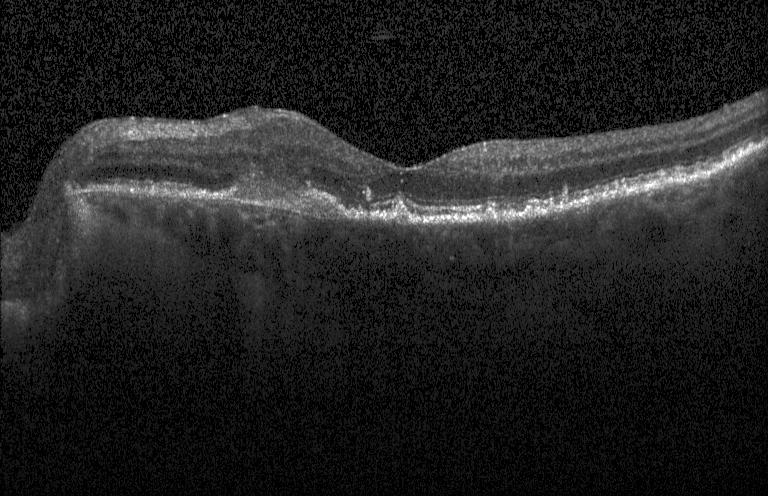 Retinal OCT cross-section
Dx: a choroidal neovascular membrane.